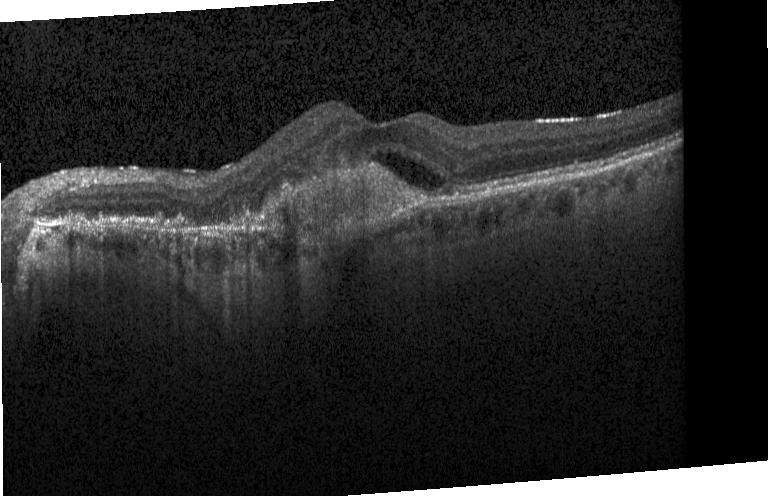
Retinal OCT B-scan.
This B-scan demonstrates choroidal neovascularization (CNV).